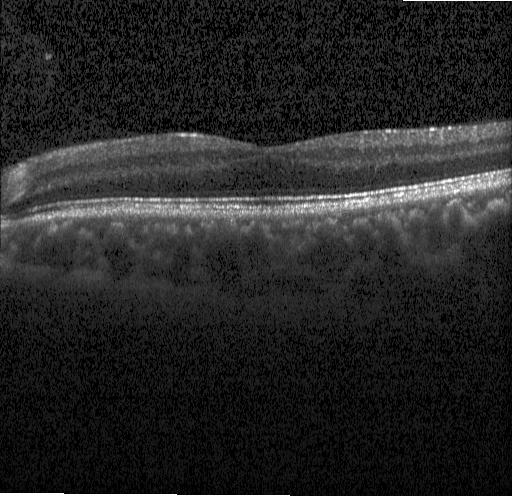
No choroidal neovascularization, diabetic macular edema, or drusen.